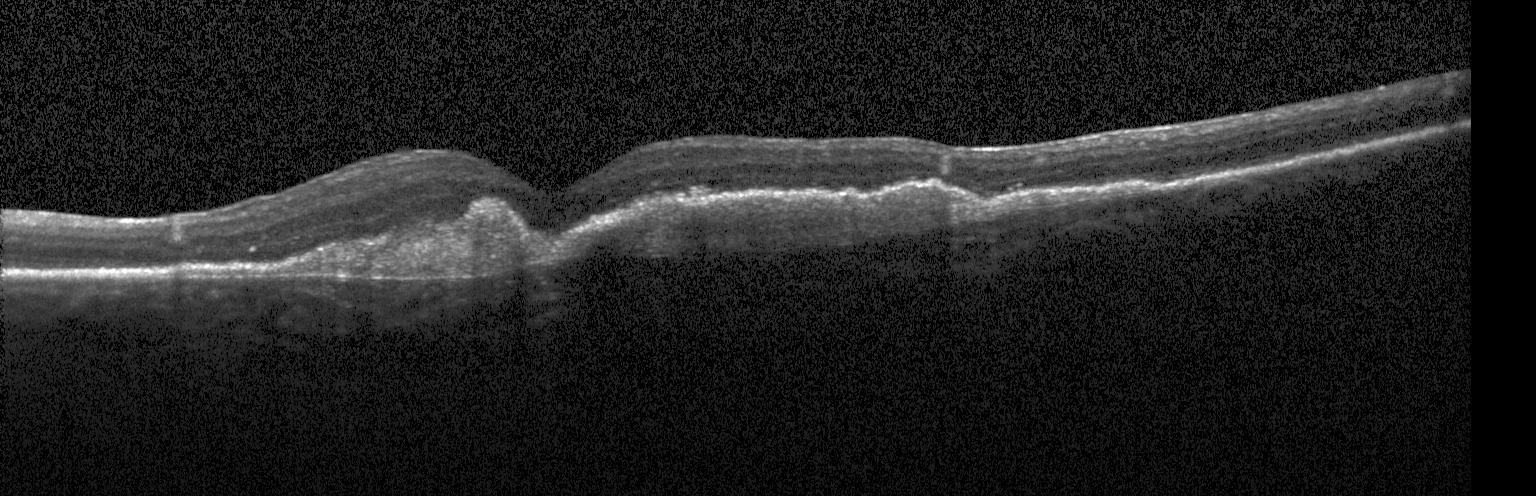 Retinal OCT B-scan · Heidelberg Spectralis OCT system. Finding: choroidal neovascularization.